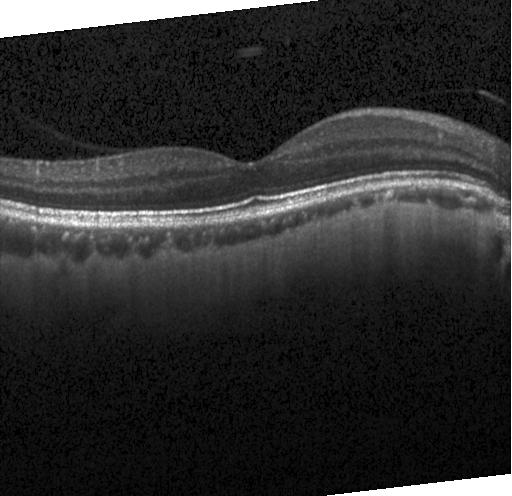 Heidelberg Spectralis OCT system. Optical coherence tomography B-scan. Through the macula
Assessment: no evidence of choroidal neovascularization, diabetic macular edema, or drusen.